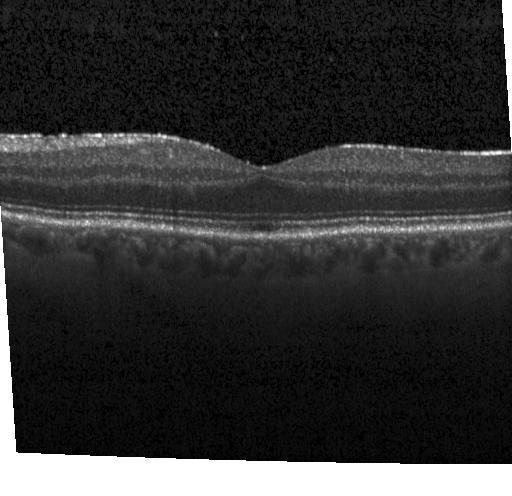
Optical coherence tomography B-scan.
Diagnosis: no choroidal neovascularization, diabetic macular edema, or drusen.